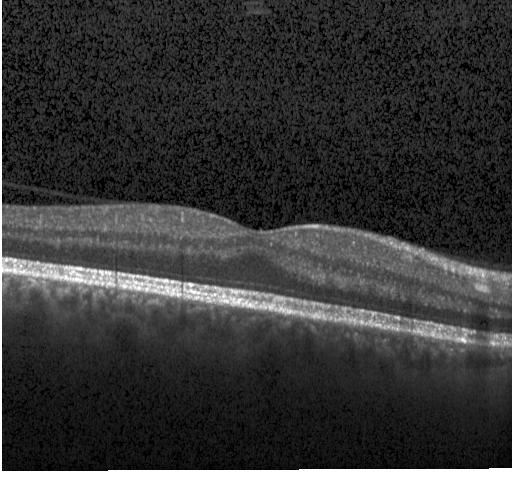 Optical coherence tomography B-scan.
Impression: no evidence of choroidal neovascularization, diabetic macular edema, or drusen.